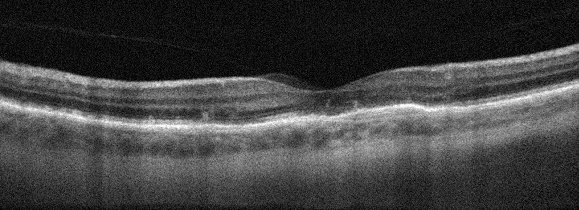 Acquired on an Optovue Avanti RTVue XR. Through the macula. Oculus sinister. Optical coherence tomography scan — Macular OCT: age-related macular degeneration.